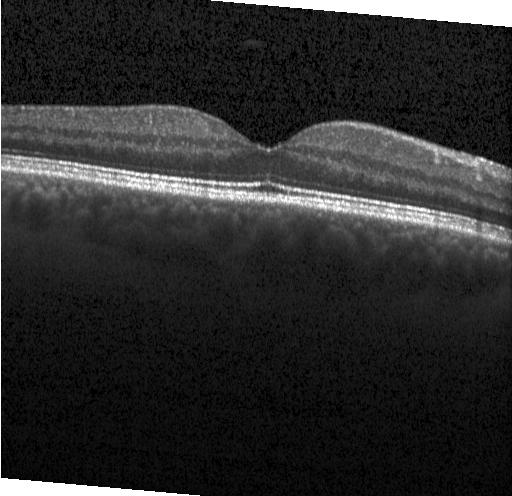
Diagnosis: no choroidal neovascularization, no diabetic macular edema, and no drusen.